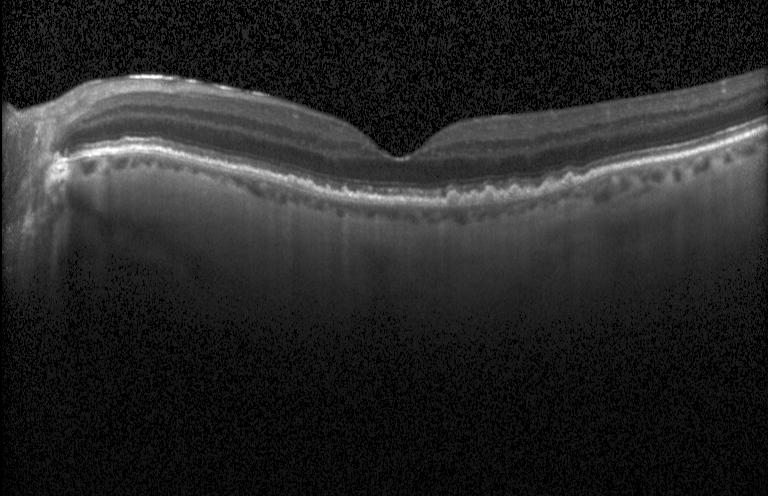 Macular OCT: drusen.